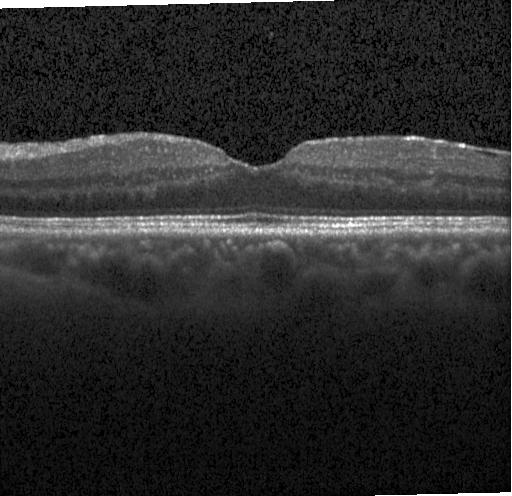
Centered on the fovea. OCT line scan. Instrument: Heidelberg Spectralis. SD-OCT. Diagnosis: no evidence of choroidal neovascularization, diabetic macular edema, or drusen.